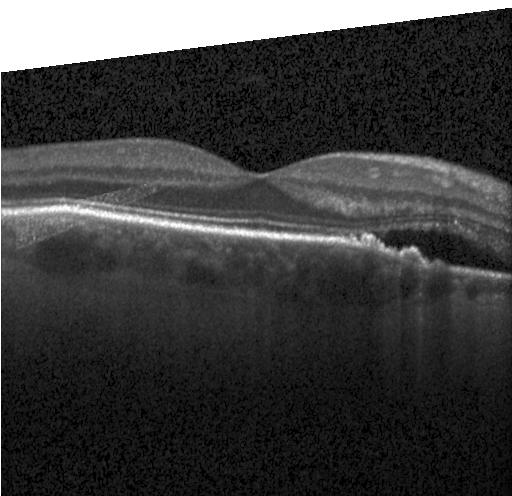
OCT line scan — CNV.